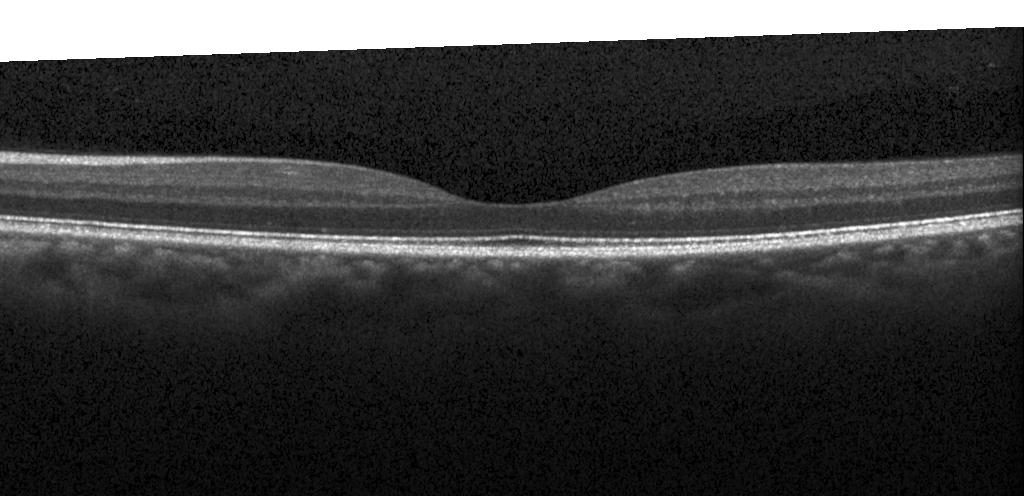
Finding: no choroidal neovascularization, diabetic macular edema, or drusen.